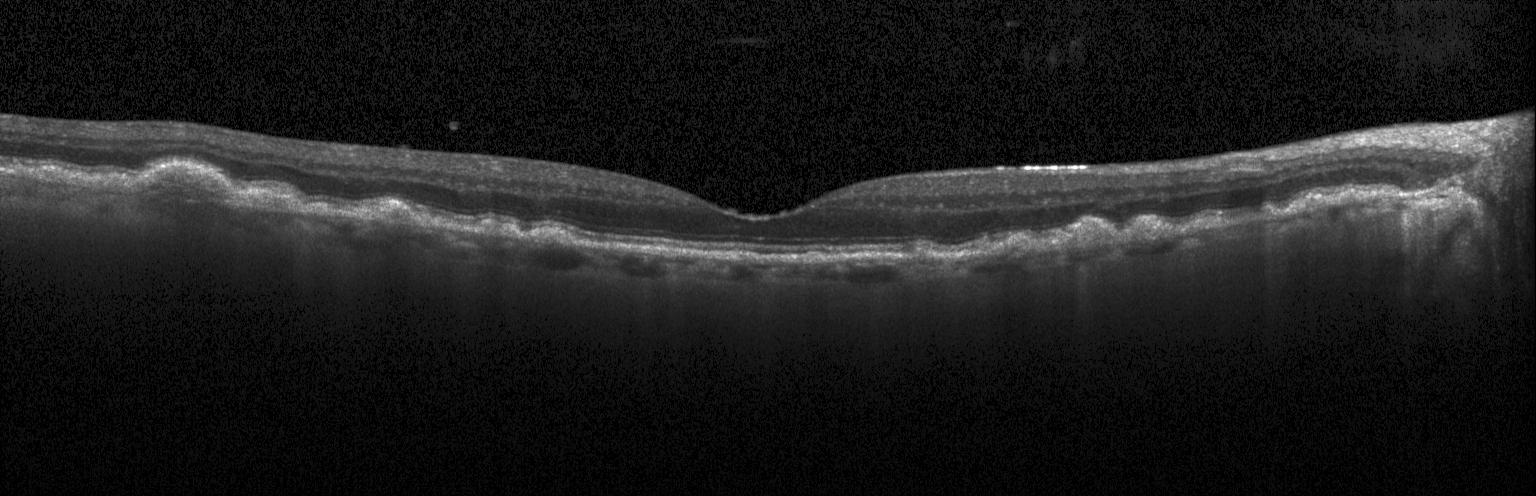

Through the macula. OCT line scan.
Diagnosis: sub-RPE drusenoid deposits.